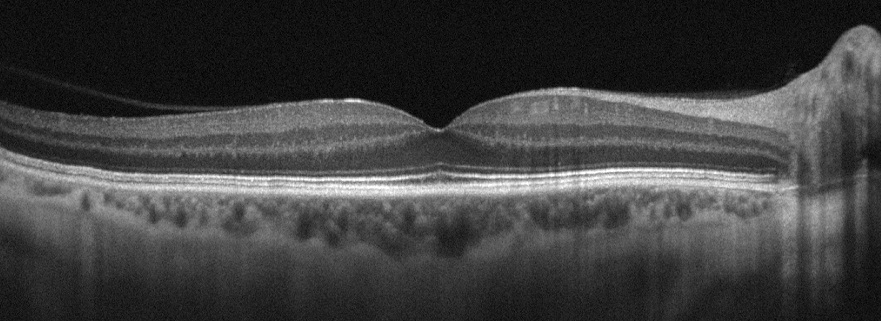 Optovue Avanti RTVue XR, optical coherence tomography scan.
The scan shows absence of AMD, DME, ERM, RAO, RVO, and vitreomacular interface disease.